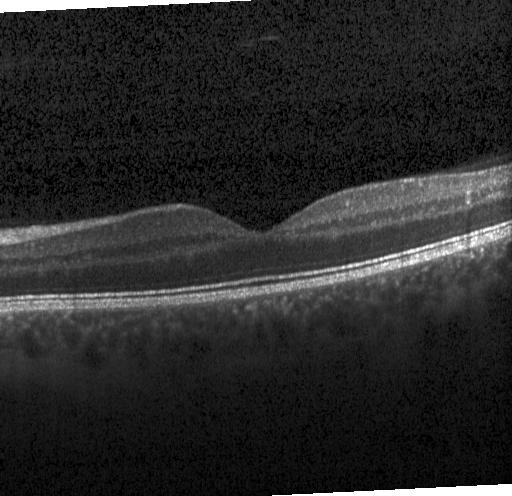
OCT B-scan showing no evidence of choroidal neovascularization, diabetic macular edema, or drusen.